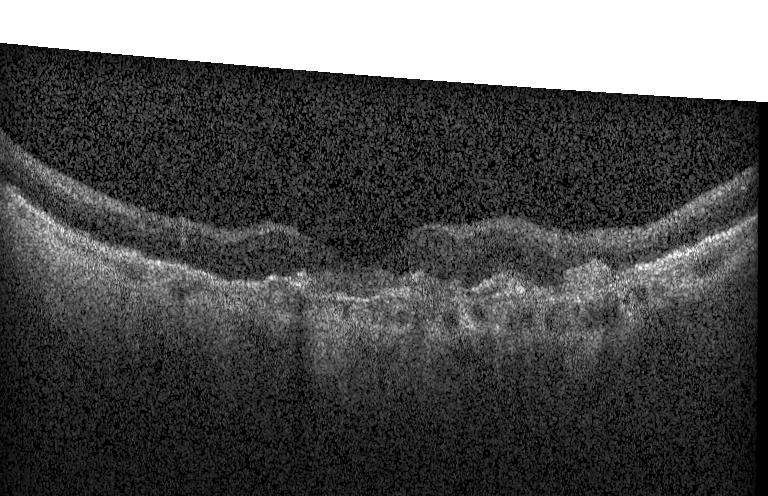
The scan shows choroidal neovascularization (CNV).